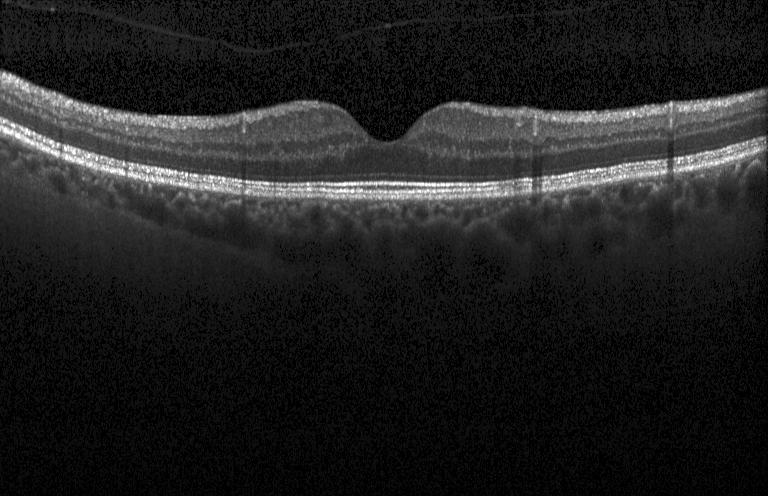
Fovea-centered; optical coherence tomography B-scan — Macular OCT: neither choroidal neovascularization, diabetic macular edema, nor drusen.